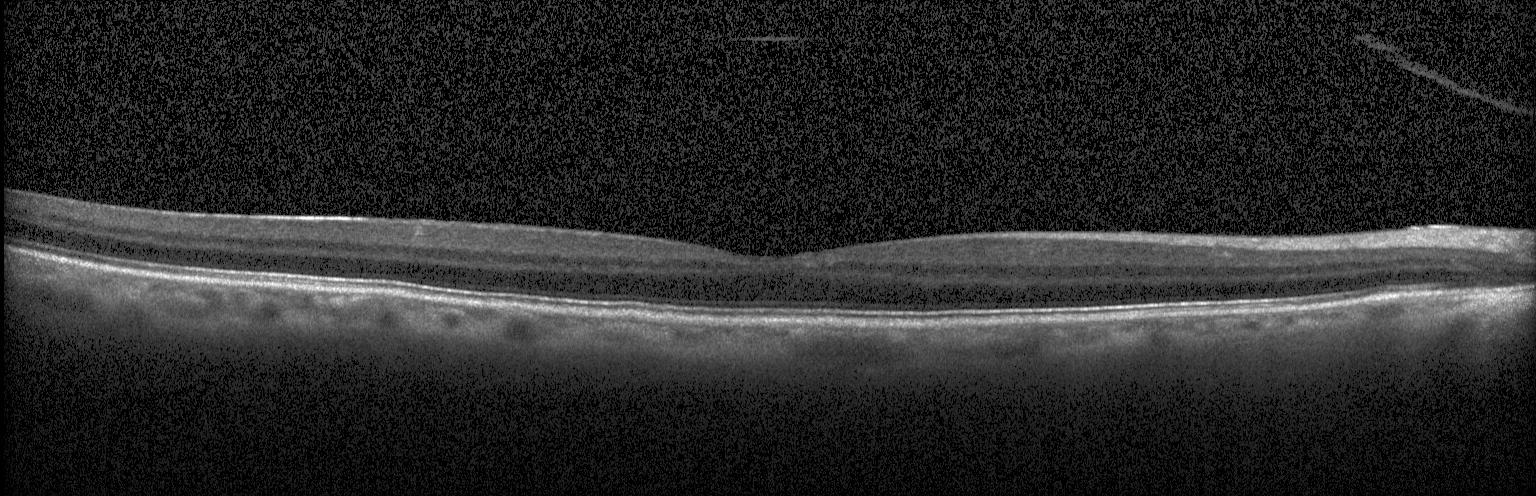
Impression: neither choroidal neovascularization, diabetic macular edema, nor drusen.